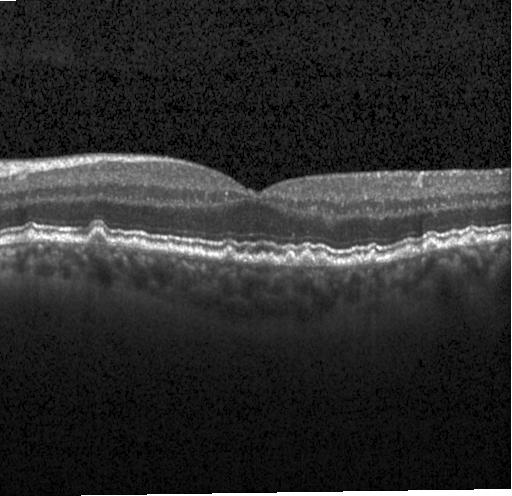 Retinal OCT cross-section — Finding: drusen.